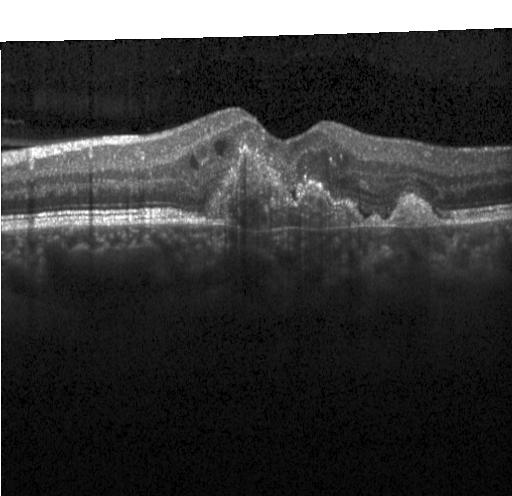
OCT B-scan showing a choroidal neovascular membrane.